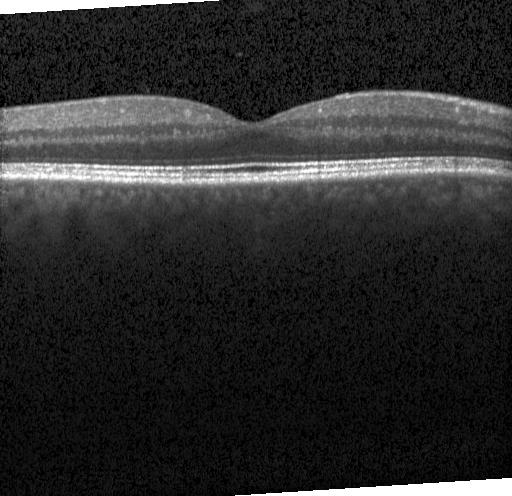

Spectral-domain OCT · fovea-centered · optical coherence tomography B-scan · instrument: Heidelberg Spectralis.
Diagnosis: no choroidal neovascularization, no diabetic macular edema, and no drusen.